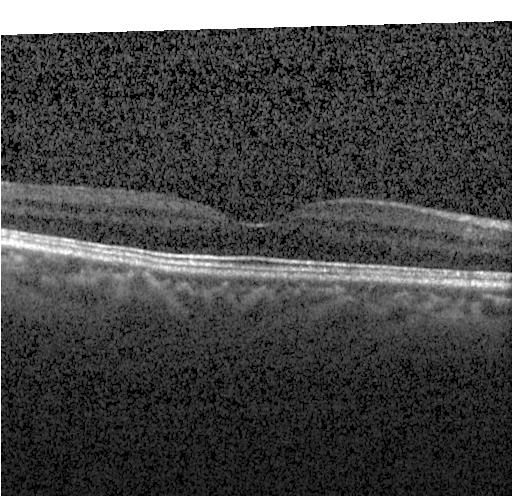 Acquired on a Heidelberg Spectralis, optical coherence tomography B-scan
Finding: no choroidal neovascularization, diabetic macular edema, or drusen.